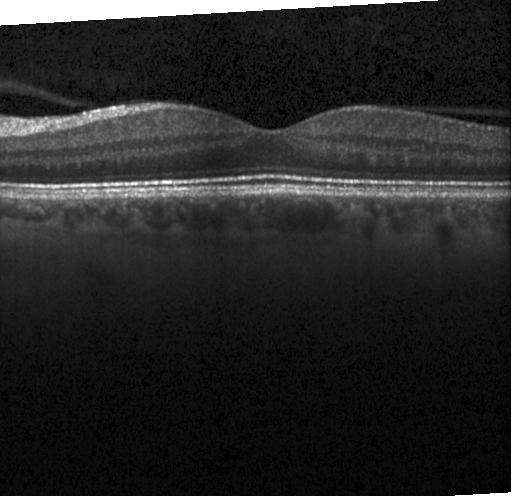 Retinal OCT cross-section.
No choroidal neovascularization, diabetic macular edema, or drusen.